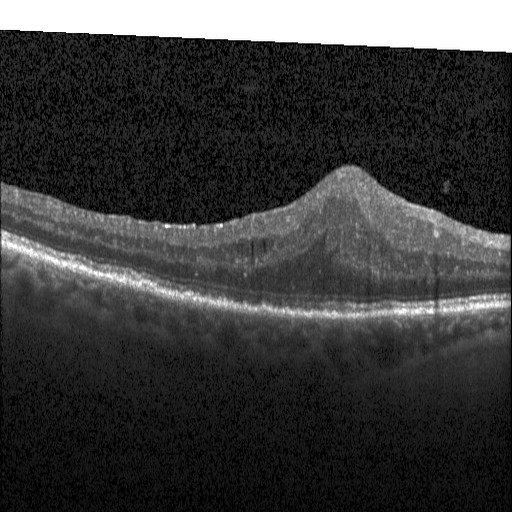

Spectral-domain optical coherence tomography · retinal OCT cross-section · macular scan — Diabetic macular edema (DME).